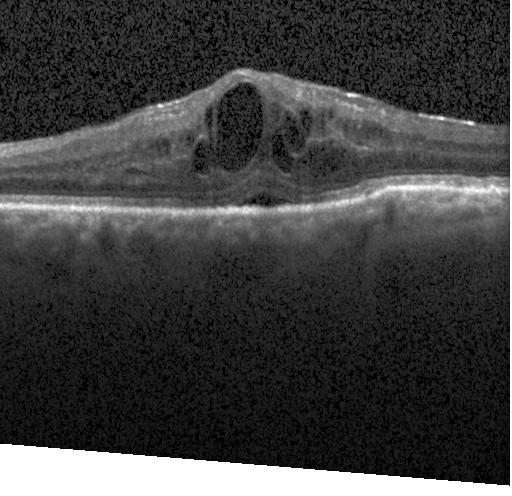

Retinal OCT B-scan. Assessment: diabetic macular edema (DME).